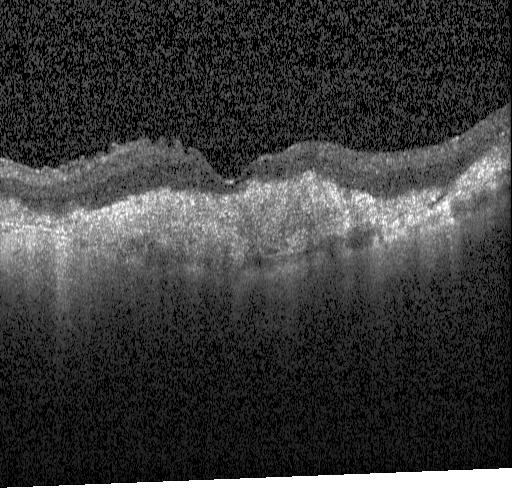 Heidelberg Spectralis OCT system, fovea-centered, optical coherence tomography scan. This B-scan demonstrates CNV.